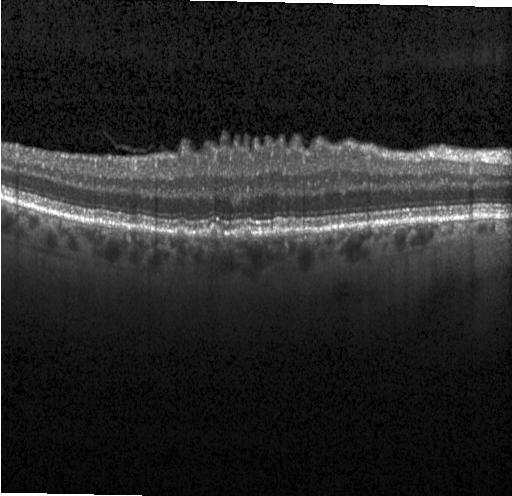 Optical coherence tomography scan, fovea-centered, spectral-domain OCT, Heidelberg Spectralis OCT system
Multiple drusen.